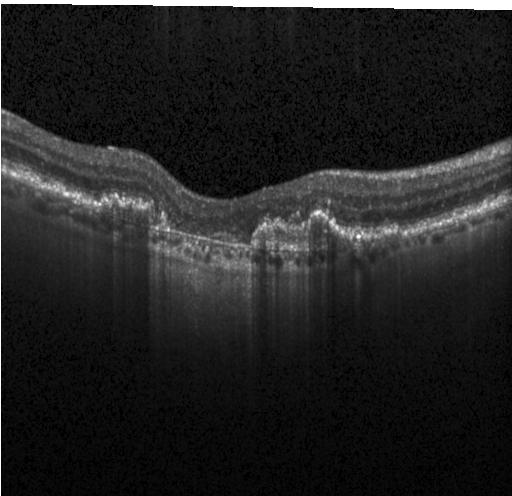 Finding: choroidal neovascularization.